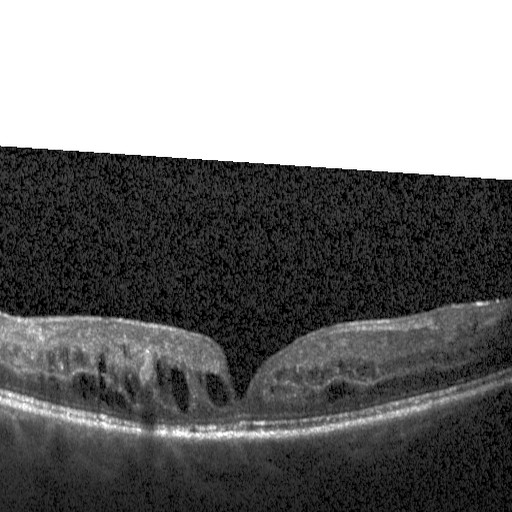

OCT B-scan showing diabetic macular edema.